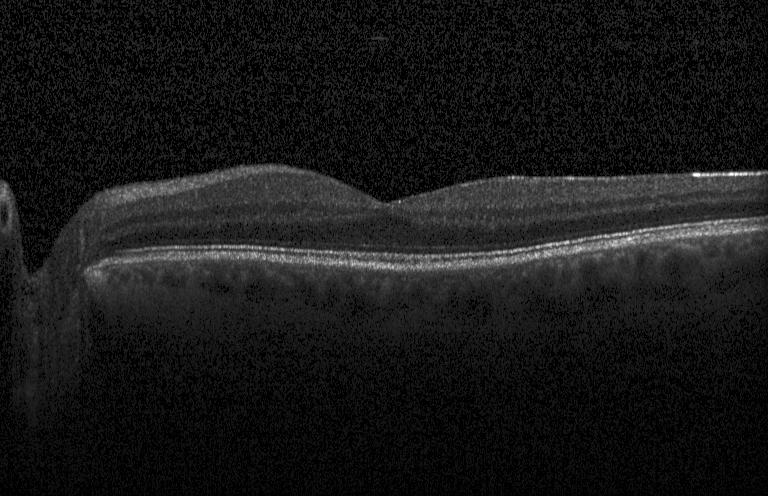
OCT scan showing neither CNV, DME, nor drusen.